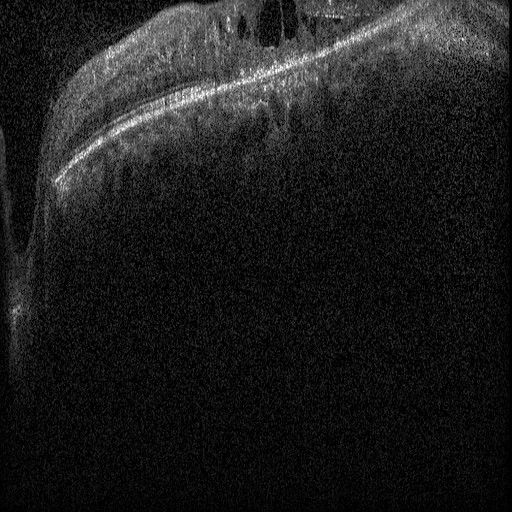 Macular OCT: diabetic macular edema.